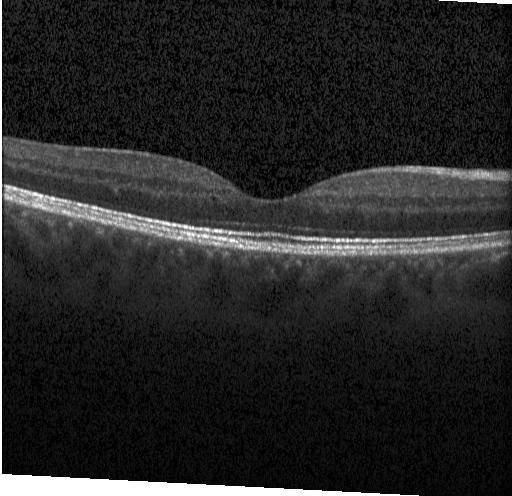 OCT finding: no choroidal neovascularization, no diabetic macular edema, and no drusen.